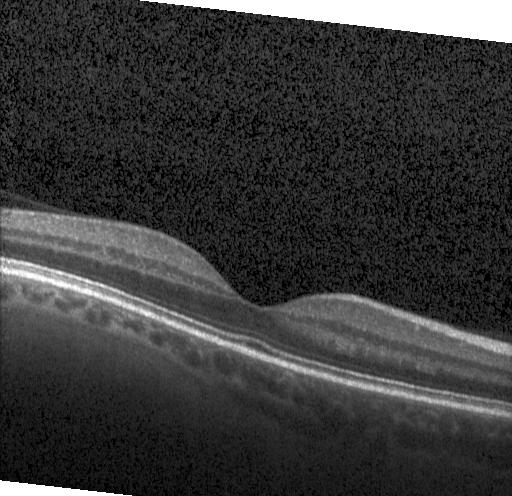
OCT line scan — Finding: no evidence of choroidal neovascularization, diabetic macular edema, or drusen.